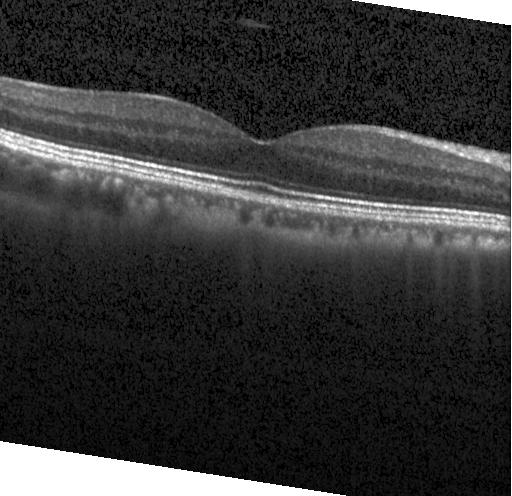

Optical coherence tomography B-scan. Spectral-domain optical coherence tomography. Instrument: Heidelberg Spectralis. Impression: no CNV, DME, or drusen.